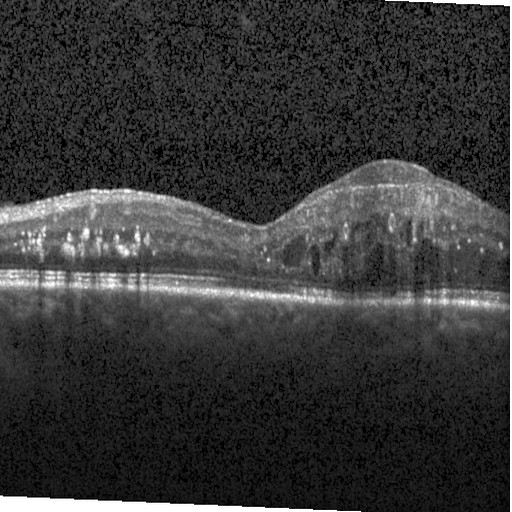

Macular OCT: diabetic macular edema.